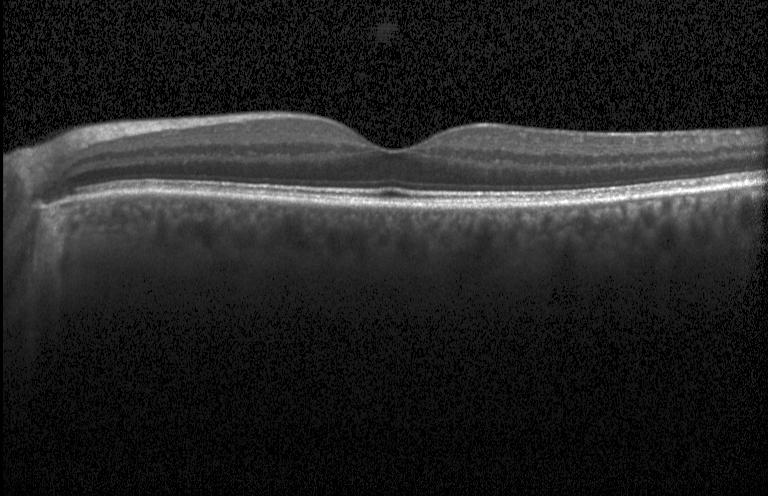 Heidelberg Spectralis · retinal OCT B-scan · macular scan.
No CNV, no DME, and no drusen.